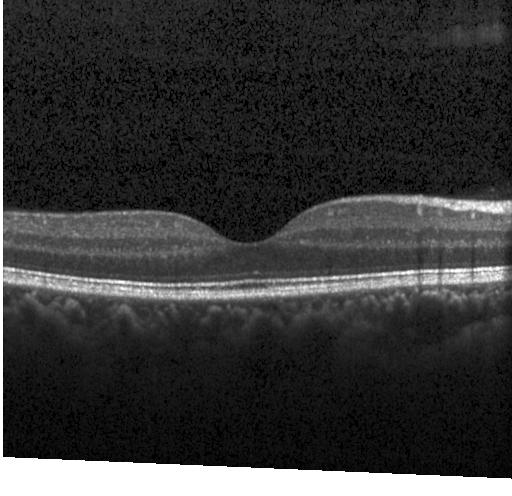

Optical coherence tomography B-scan, SD-OCT, macular scan, Heidelberg Spectralis.
Assessment: no CNV, no DME, and no drusen.